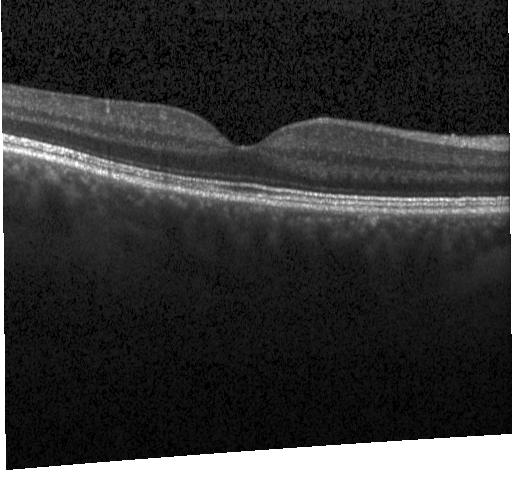 Retinal OCT B-scan
No CNV, DME, or drusen.